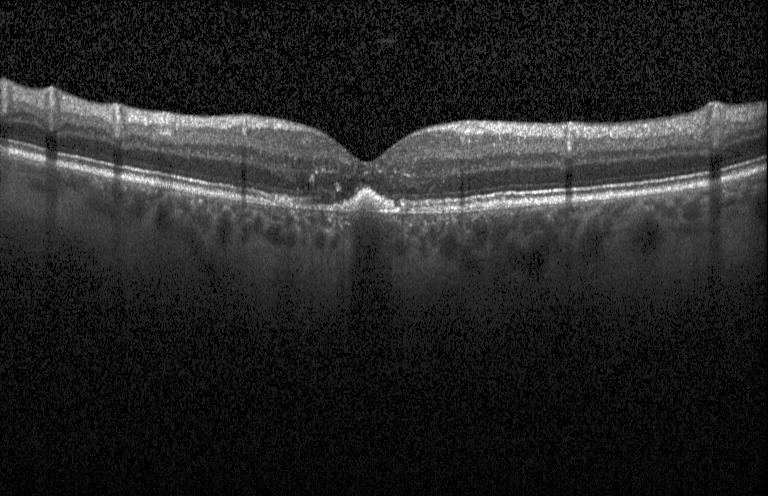

OCT line scan · centered on the fovea. Impression: choroidal neovascularization.